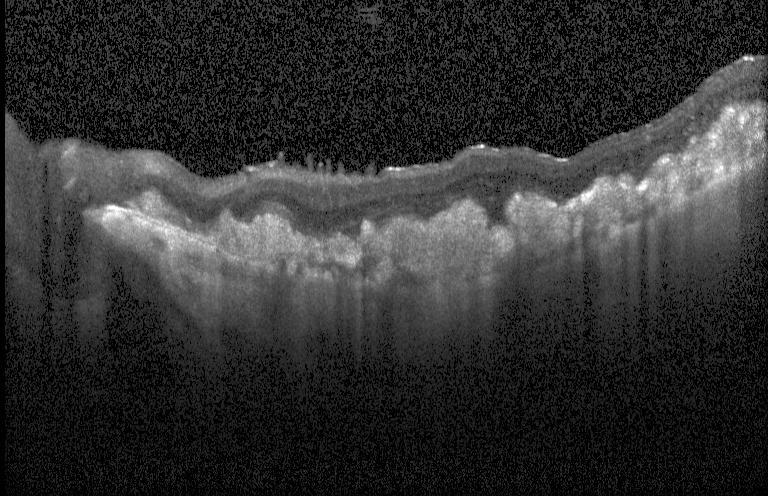

OCT line scan, centered on the fovea — OCT finding: CNV.